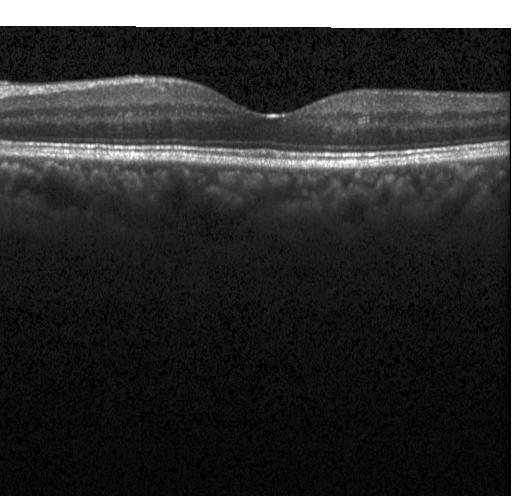 Diagnosis: no choroidal neovascularization, diabetic macular edema, or drusen.